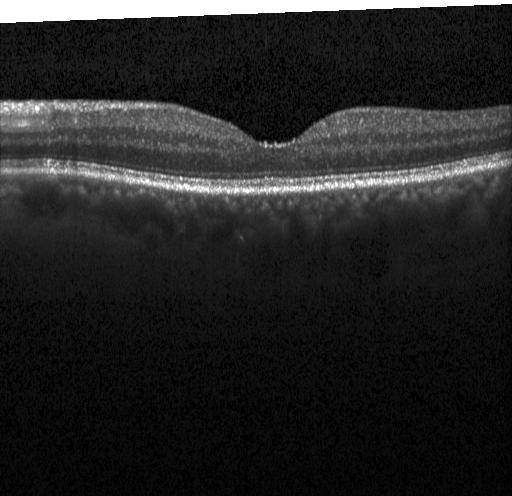 Impression: no choroidal neovascularization, no diabetic macular edema, and no drusen.